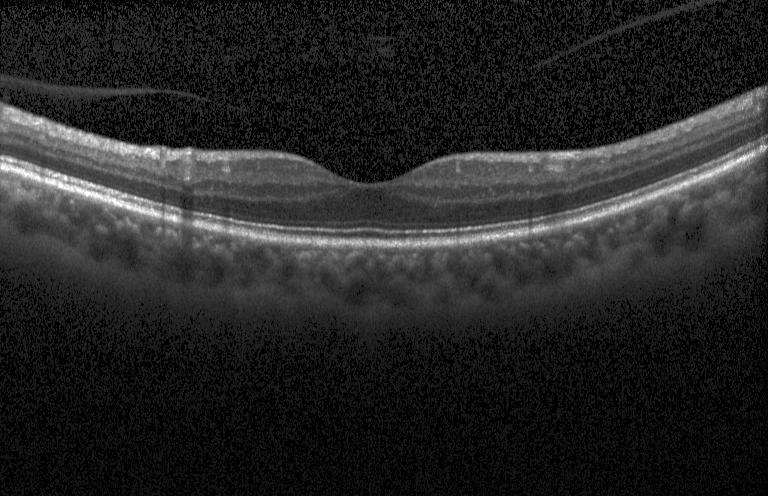 Spectral-domain OCT, retinal OCT cross-section.
Impression: no choroidal neovascularization, no diabetic macular edema, and no drusen.